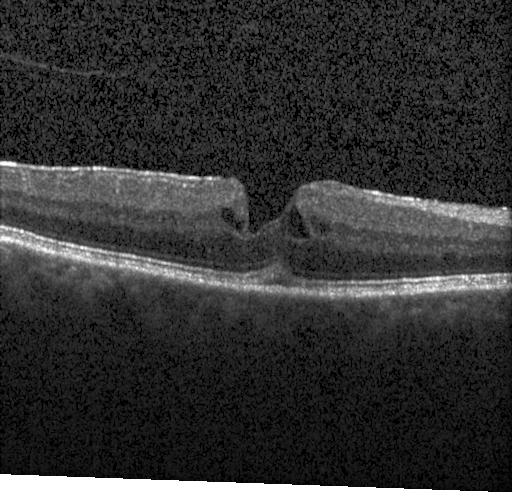 Macular OCT demonstrating DME.